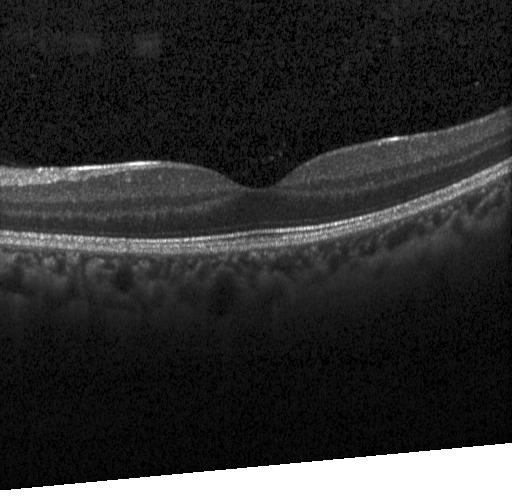

Acquired on a Heidelberg Spectralis · macular scan · OCT B-scan.
This B-scan demonstrates no choroidal neovascularization, diabetic macular edema, or drusen.